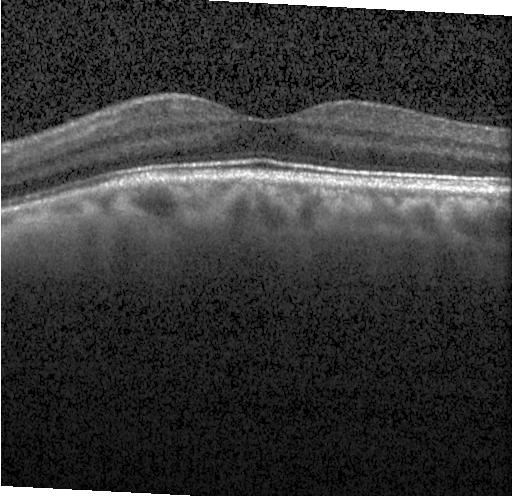
OCT B-scan showing no CNV, DME, or drusen.